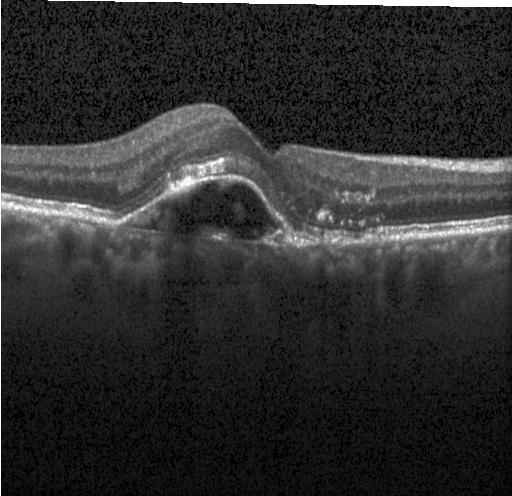 Fovea-centered, instrument: Heidelberg Spectralis, optical coherence tomography B-scan, SD-OCT — Impression: a choroidal neovascular membrane.